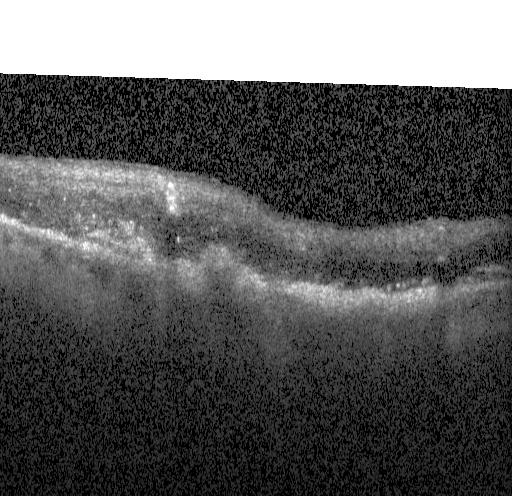
OCT line scan; Heidelberg Spectralis; SD-OCT.
Diagnosis: a choroidal neovascular membrane.